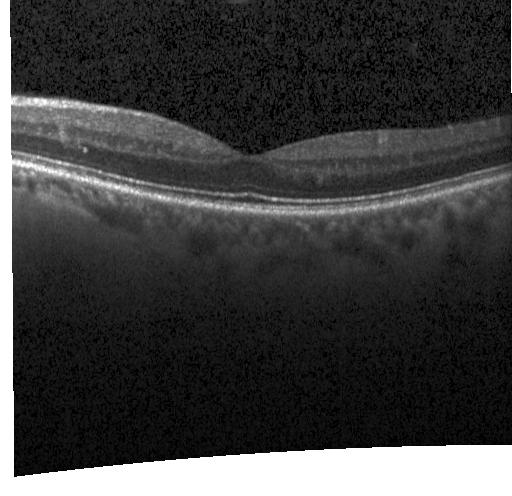

Heidelberg Spectralis OCT system · macular scan · spectral-domain OCT · OCT B-scan
Macular OCT: no choroidal neovascularization, diabetic macular edema, or drusen.